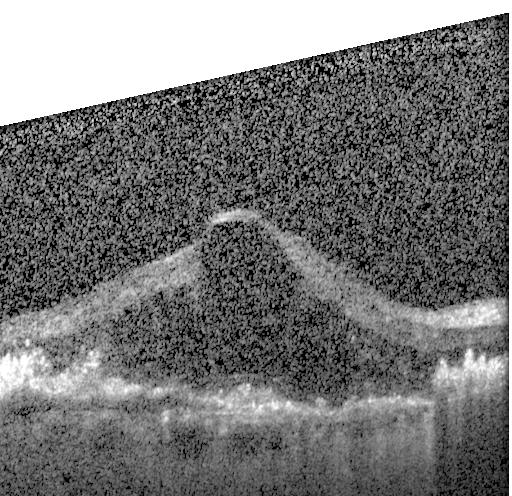

OCT line scan
Dx: a choroidal neovascular membrane.